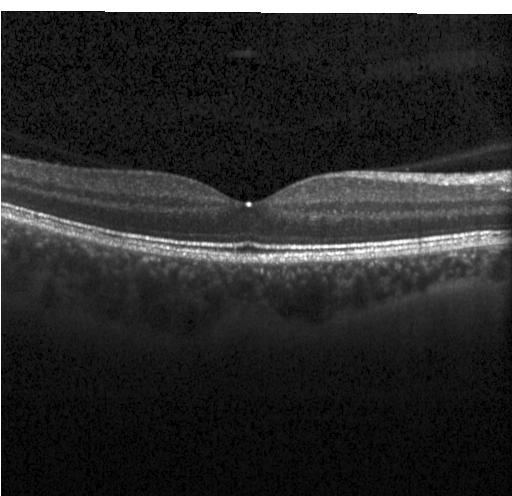 Optical coherence tomography B-scan. The scan shows no choroidal neovascularization, diabetic macular edema, or drusen.